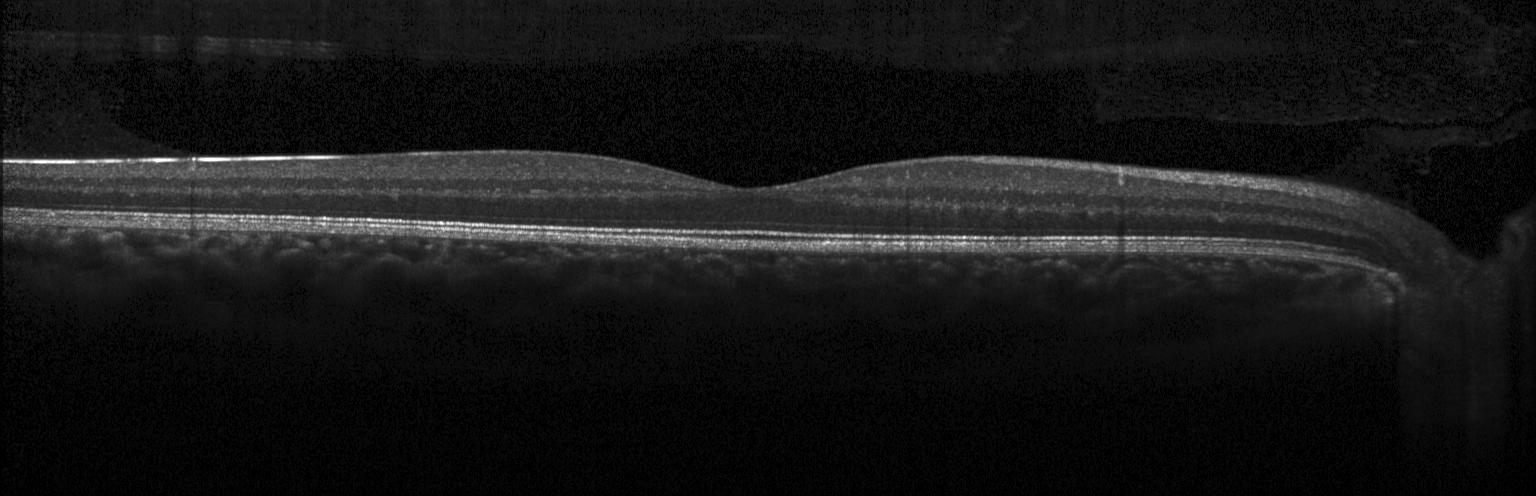 Acquired on a Heidelberg Spectralis; OCT B-scan; horizontal scan through the fovea; spectral-domain optical coherence tomography
No choroidal neovascularization, diabetic macular edema, or drusen.